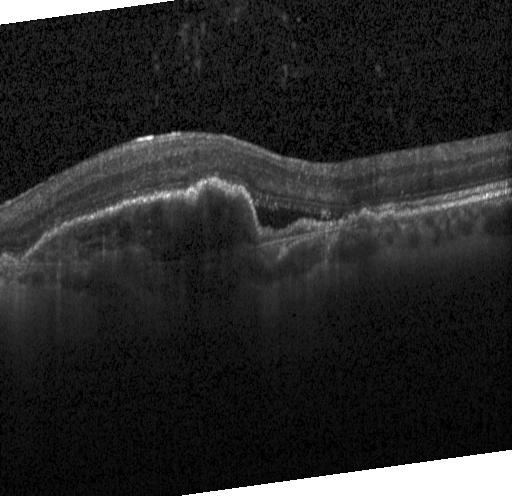 Retinal OCT cross-section. This B-scan demonstrates choroidal neovascularization (CNV).